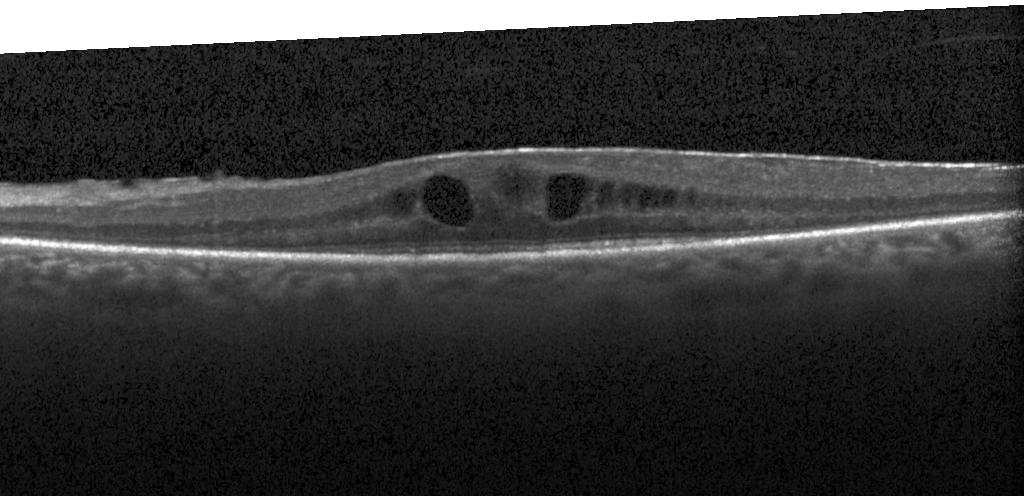
Diabetic macular edema (DME).